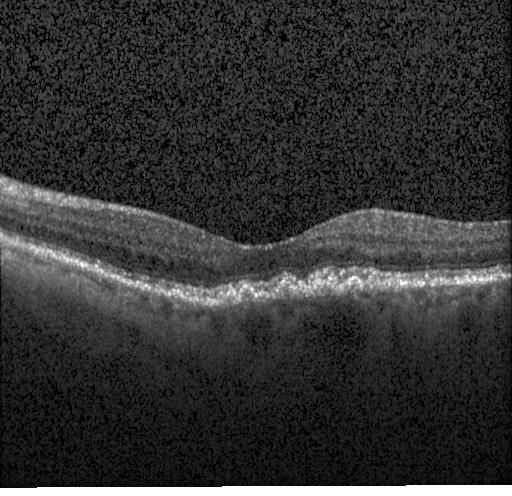
Retinal OCT cross-section. Assessment: multiple drusen.